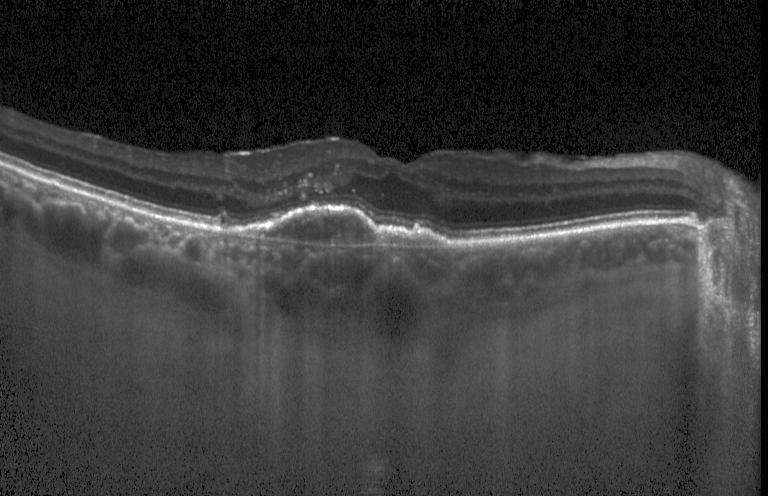
Spectral-domain OCT. Fovea-centered. Retinal OCT B-scan.
Impression: choroidal neovascularization (CNV).